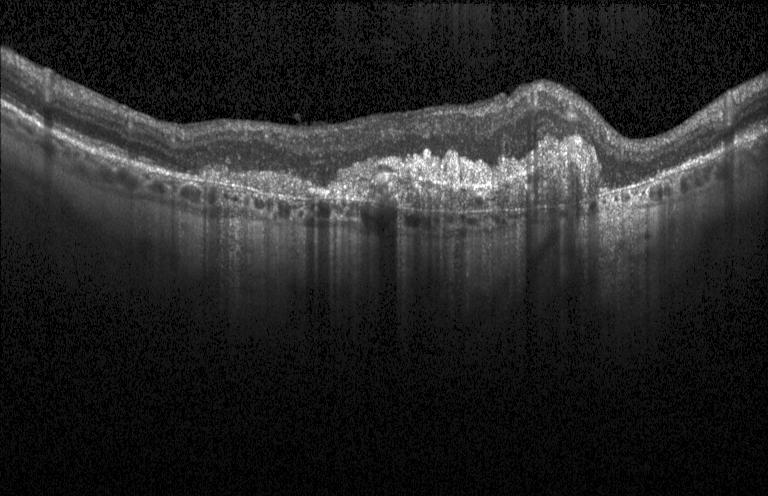
OCT line scan, SD-OCT. Dx: a choroidal neovascular membrane.